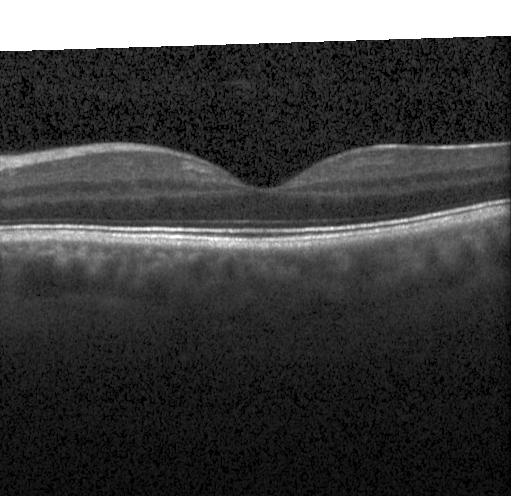

Diagnosis: no evidence of CNV, DME, or drusen.